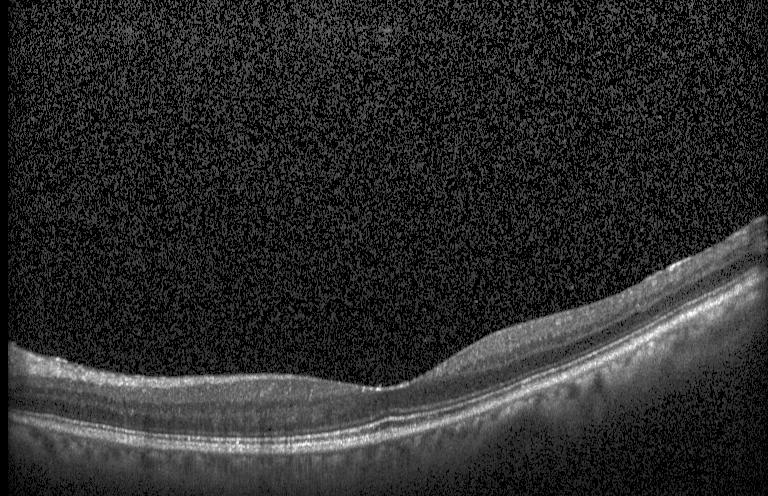

Diagnosis: no evidence of choroidal neovascularization, diabetic macular edema, or drusen.